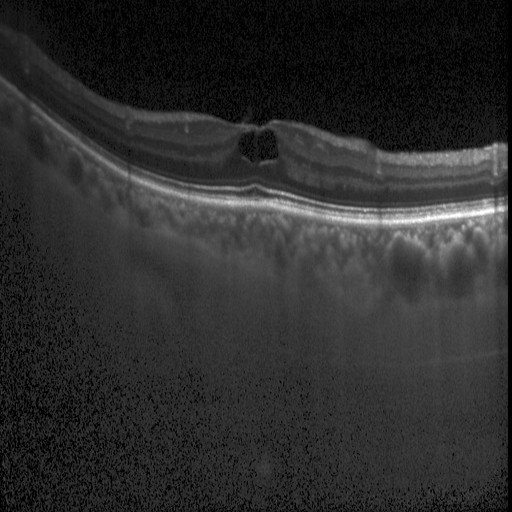 Retinal OCT B-scan; fovea-centered; instrument: Heidelberg Spectralis — This B-scan demonstrates diabetic macular edema.